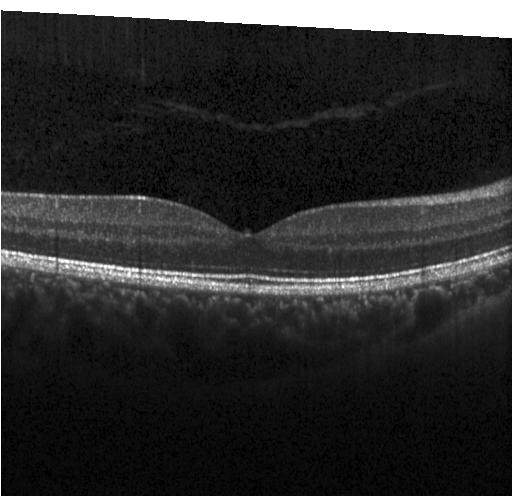

OCT line scan; SD-OCT. Assessment: no evidence of CNV, DME, or drusen.